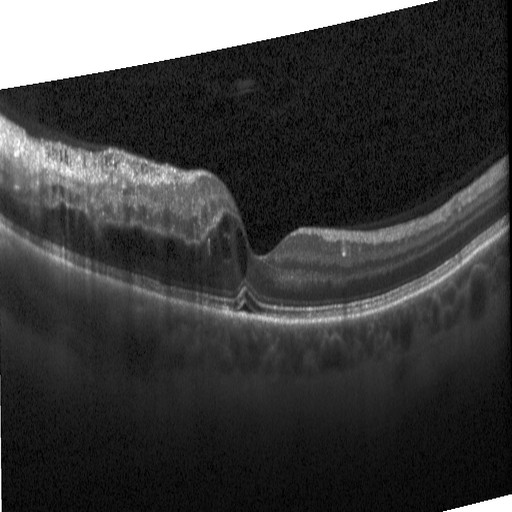 Horizontal scan through the fovea; optical coherence tomography B-scan. Dx: DME.